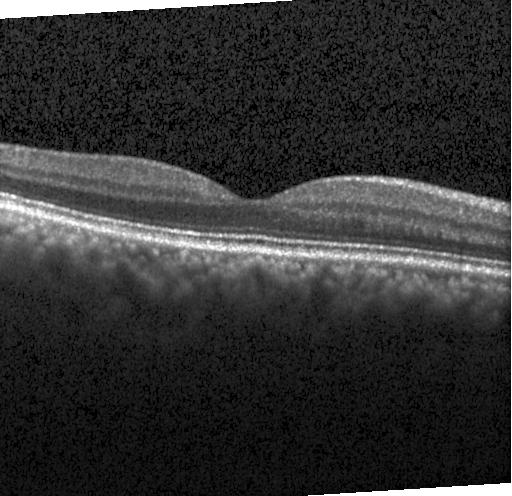
OCT finding: neither CNV, DME, nor drusen.